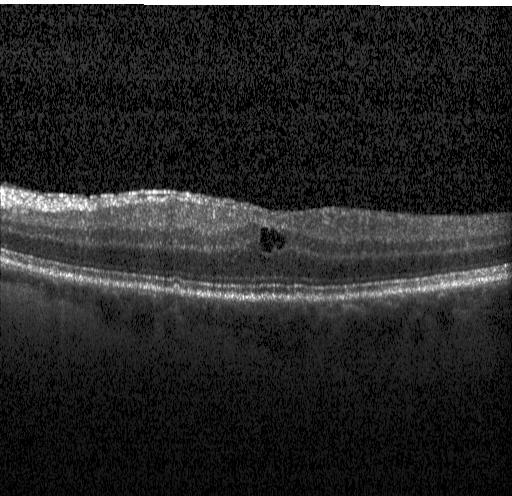 Spectral-domain optical coherence tomography, Heidelberg Spectralis, optical coherence tomography scan, through the macula. Impression: diabetic macular edema (DME).